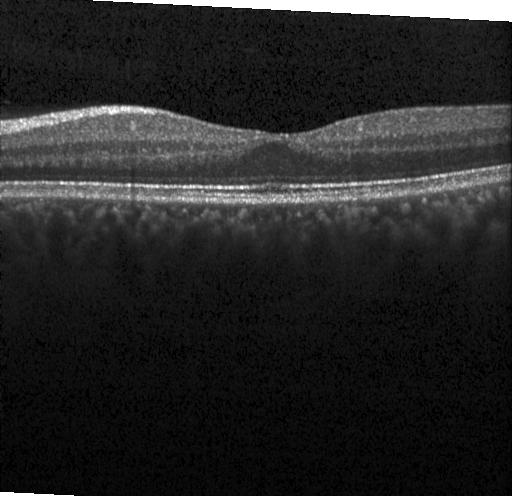
Spectral-domain OCT B-scan: no evidence of choroidal neovascularization, diabetic macular edema, or drusen.